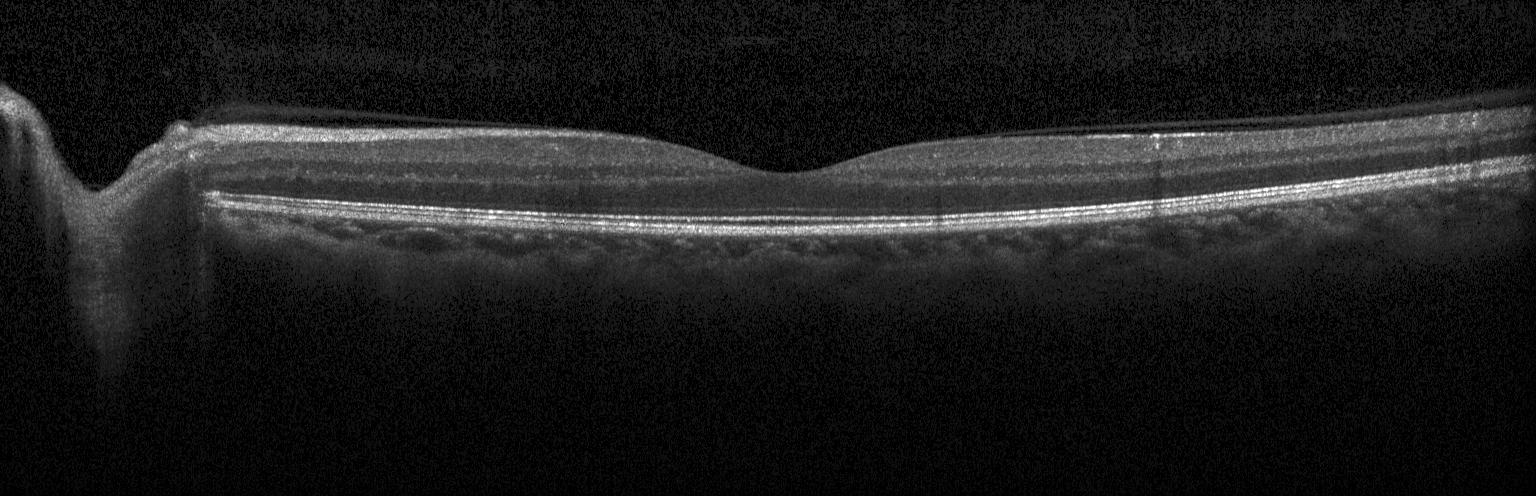
Retinal OCT cross-section; through the macula; spectral-domain optical coherence tomography
Assessment: no CNV, no DME, and no drusen.